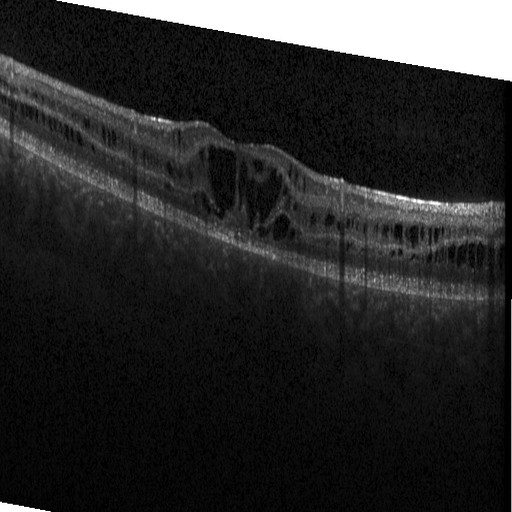

OCT line scan. This B-scan demonstrates diabetic macular edema (DME).